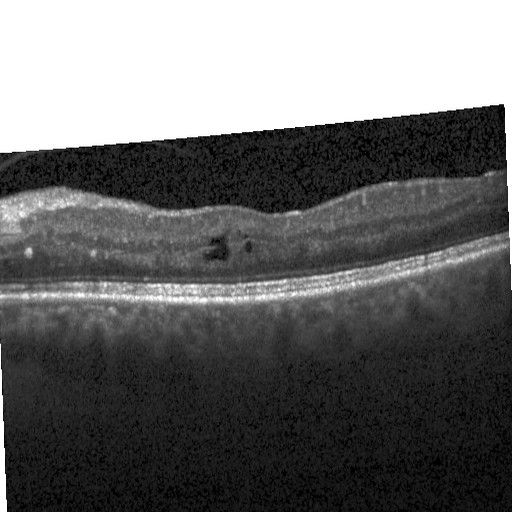
Retinal OCT B-scan · spectral-domain optical coherence tomography — Finding: diabetic macular edema.